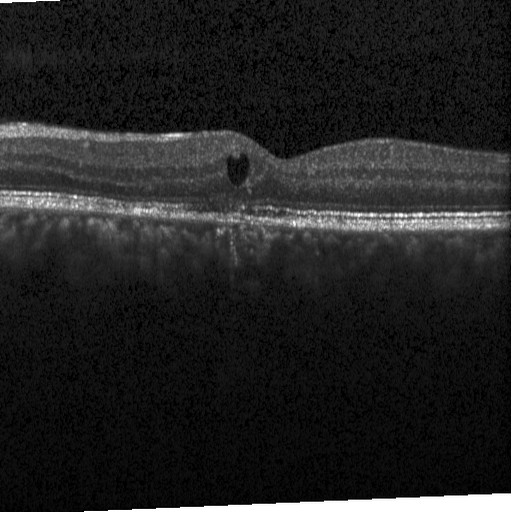

OCT line scan · instrument: Heidelberg Spectralis · spectral-domain OCT · horizontal scan through the fovea. The scan shows diabetic macular edema (DME).